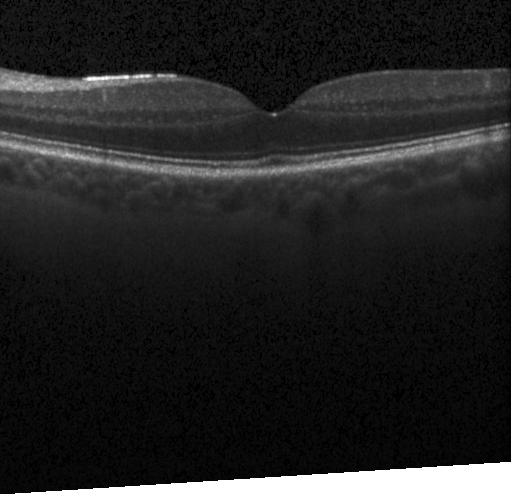

Spectral-domain OCT. Horizontal scan through the fovea. Retinal OCT cross-section. Acquired on a Heidelberg Spectralis
Finding: no CNV, DME, or drusen.